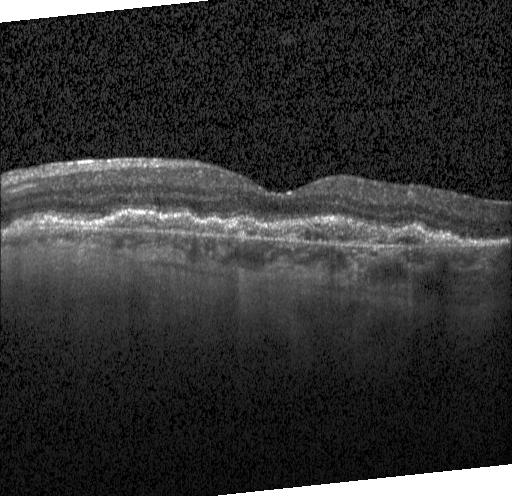

OCT line scan — Finding: a choroidal neovascular membrane.